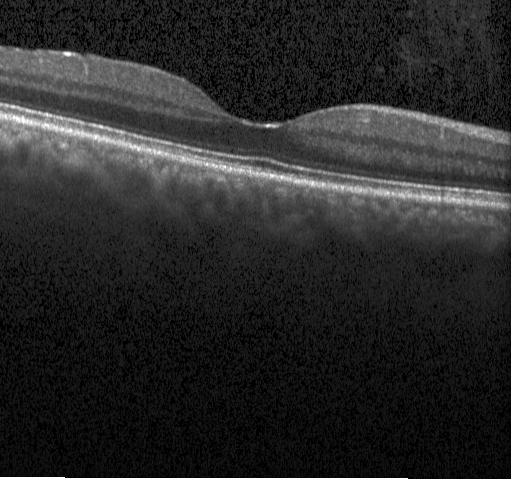
Heidelberg Spectralis OCT system; retinal OCT cross-section; through the macula
Diagnosis: no evidence of choroidal neovascularization, diabetic macular edema, or drusen.